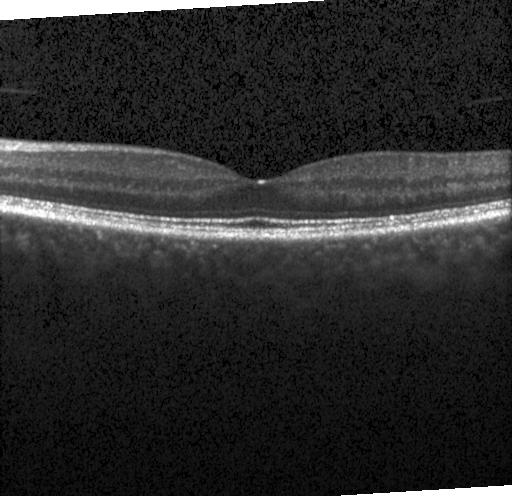

Retinal OCT B-scan
Finding: neither CNV, DME, nor drusen.